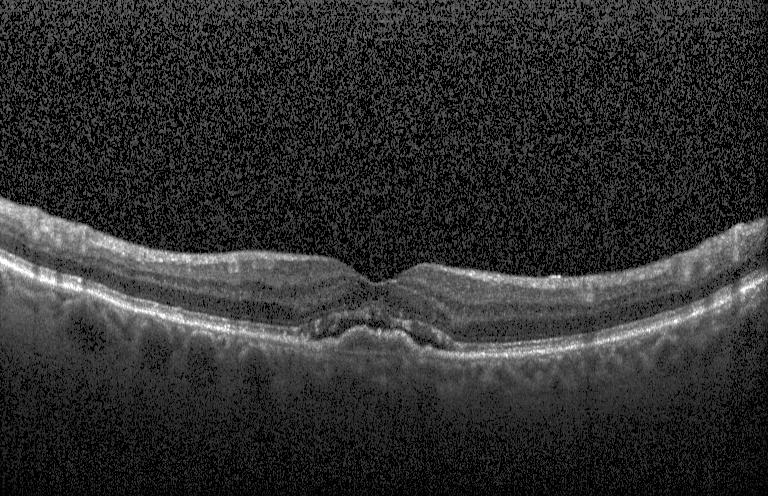

OCT B-scan. Spectral-domain optical coherence tomography.
The scan shows CNV.